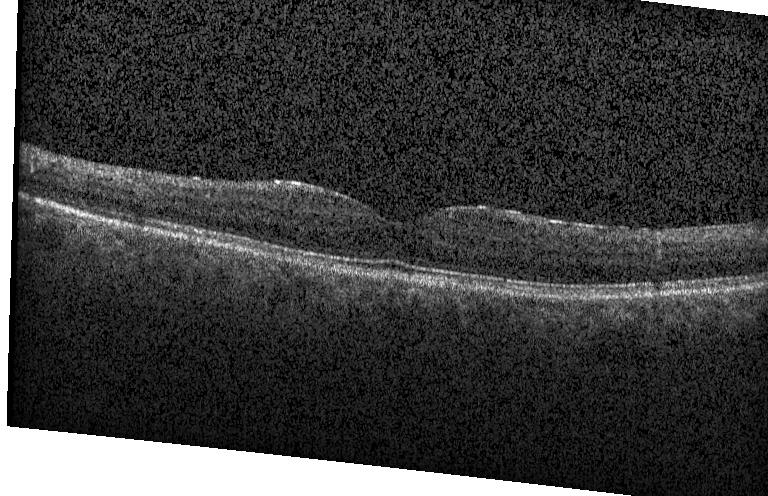

Optical coherence tomography B-scan, macular scan.
Diagnosis: no CNV, DME, or drusen.